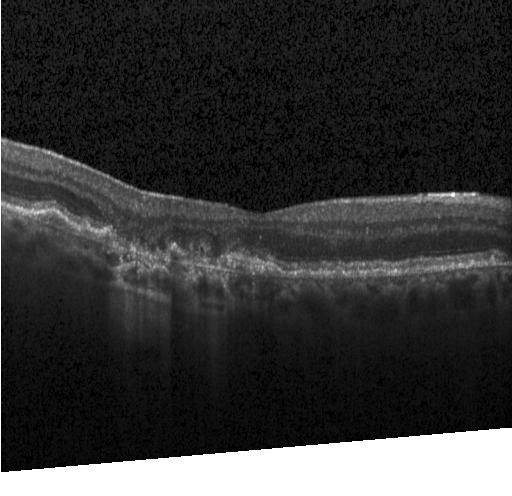 Retinal OCT cross-section; acquired on a Heidelberg Spectralis.
OCT finding: a choroidal neovascular membrane.